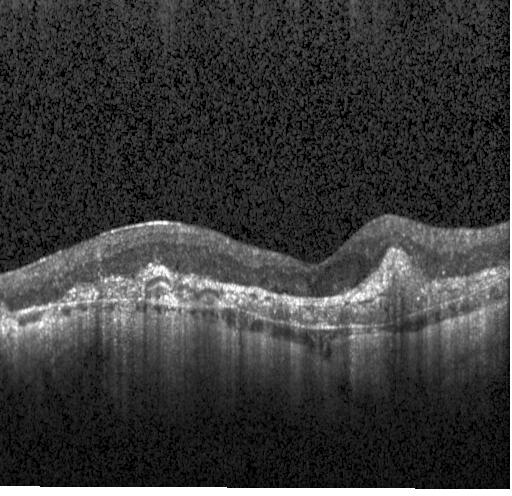

Heidelberg Spectralis. Fovea-centered. Optical coherence tomography scan.
Diagnosis: a choroidal neovascular membrane.